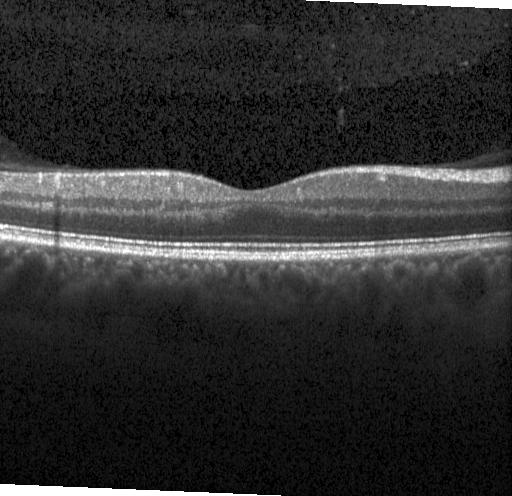

Impression: no choroidal neovascularization, diabetic macular edema, or drusen.